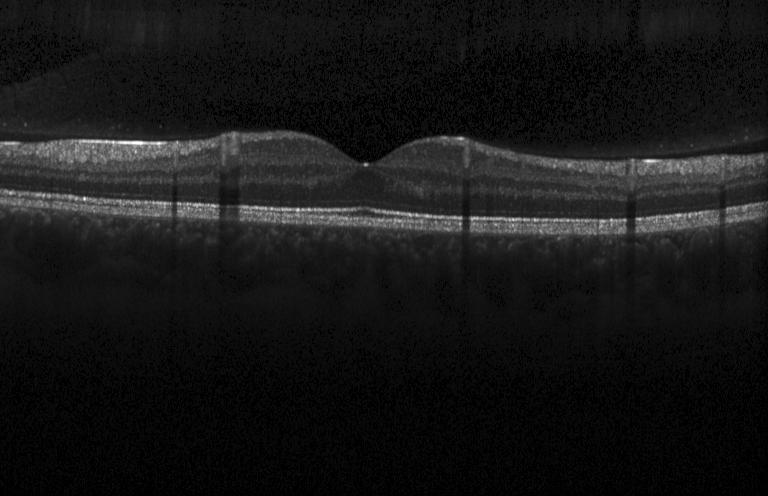
Heidelberg Spectralis, retinal OCT B-scan — Diagnosis: no choroidal neovascularization, diabetic macular edema, or drusen.